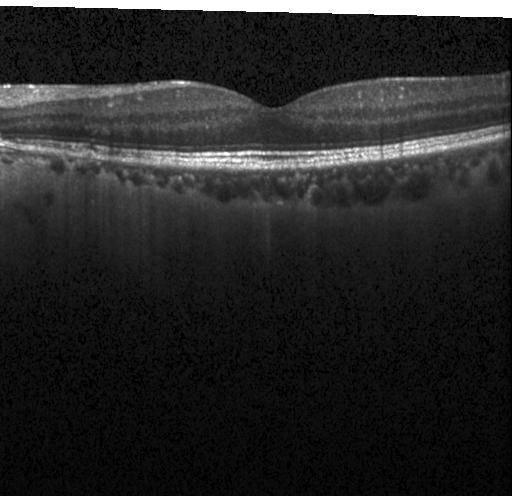

Optical coherence tomography scan, Heidelberg Spectralis, spectral-domain optical coherence tomography, macular scan — Macular OCT: no choroidal neovascularization, no diabetic macular edema, and no drusen.